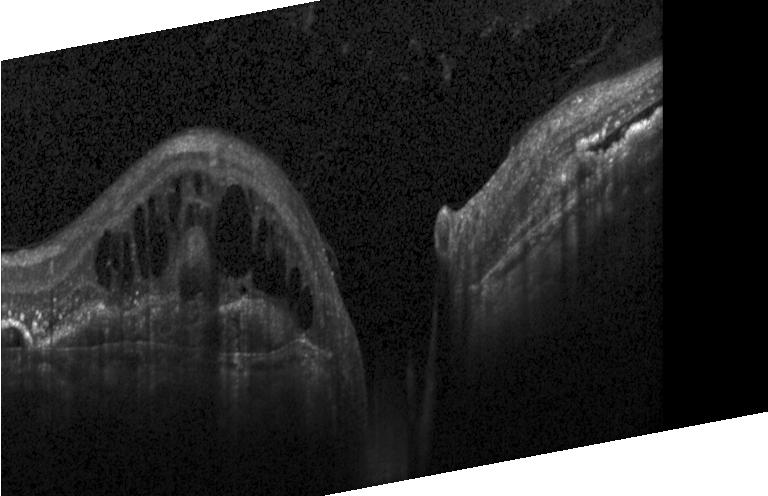
Finding: CNV.